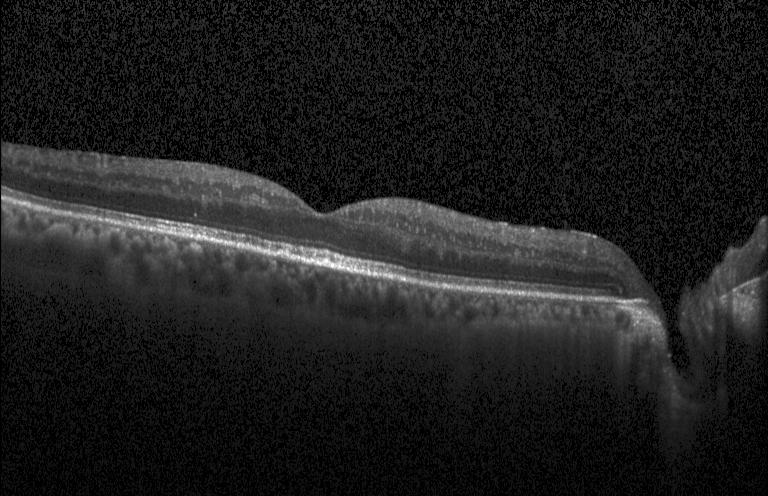
Dx: no evidence of choroidal neovascularization, diabetic macular edema, or drusen.